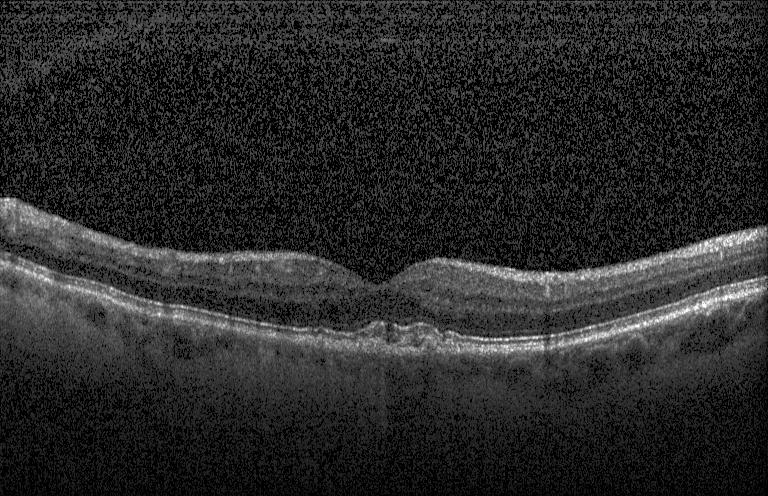

Finding: choroidal neovascularization (CNV).